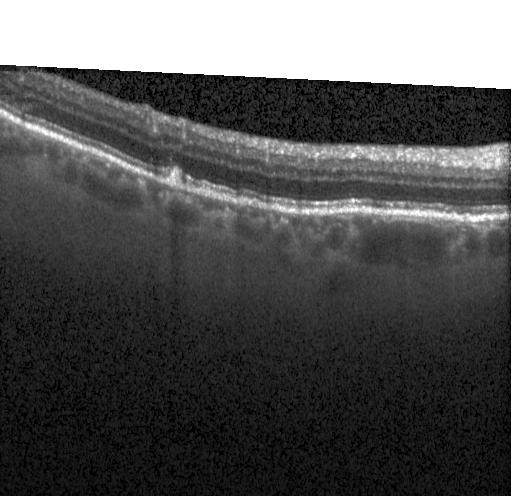
Spectral-domain optical coherence tomography. Heidelberg Spectralis. Retinal OCT cross-section. Centered on the fovea. Impression: sub-RPE drusenoid deposits.